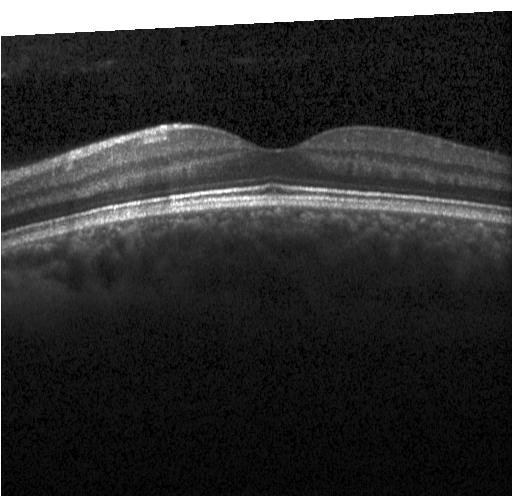
The scan shows no evidence of CNV, DME, or drusen.